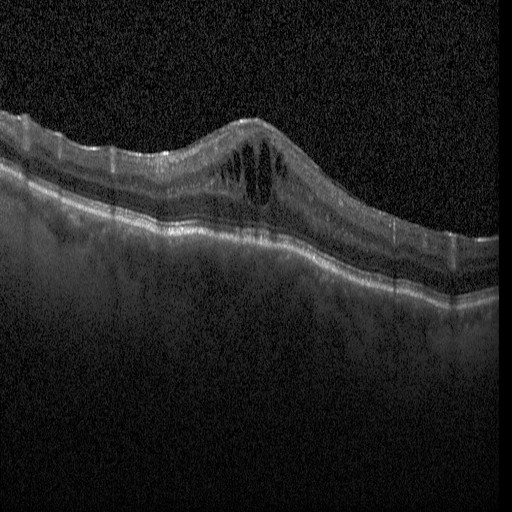
OCT line scan, acquired on a Heidelberg Spectralis
This B-scan demonstrates diabetic macular edema.